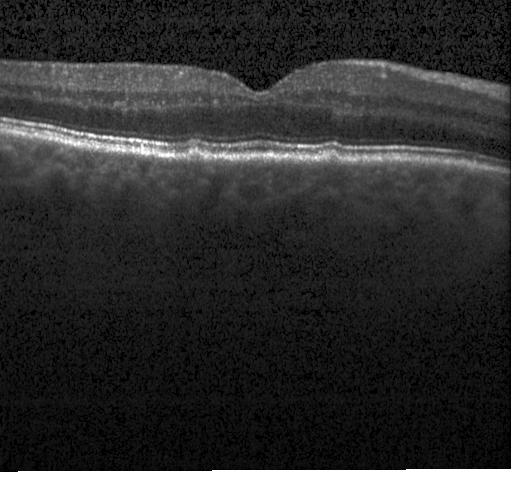 Assessment: drusen.